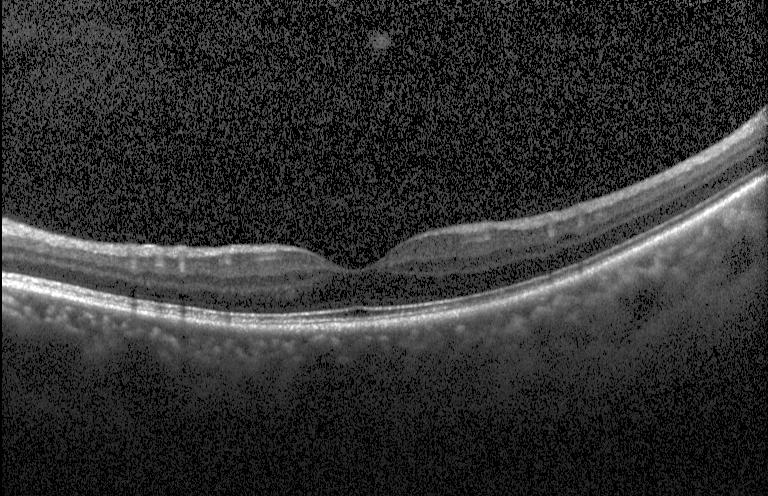
Retinal OCT B-scan
This B-scan demonstrates no CNV, no DME, and no drusen.